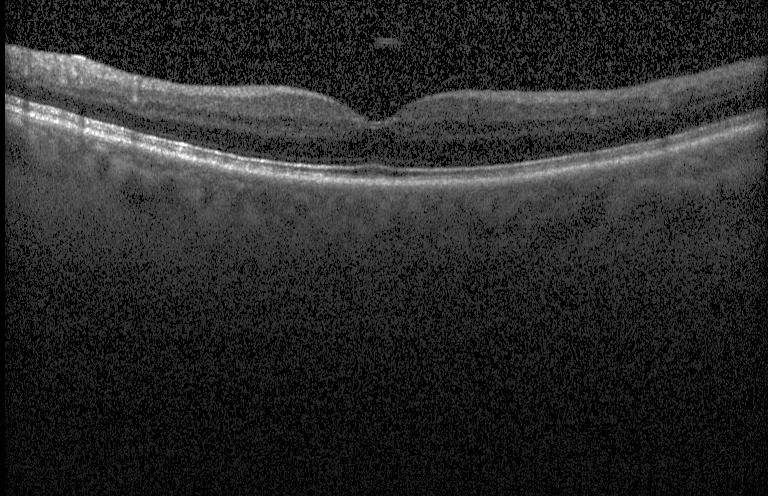

Finding: no evidence of CNV, DME, or drusen.